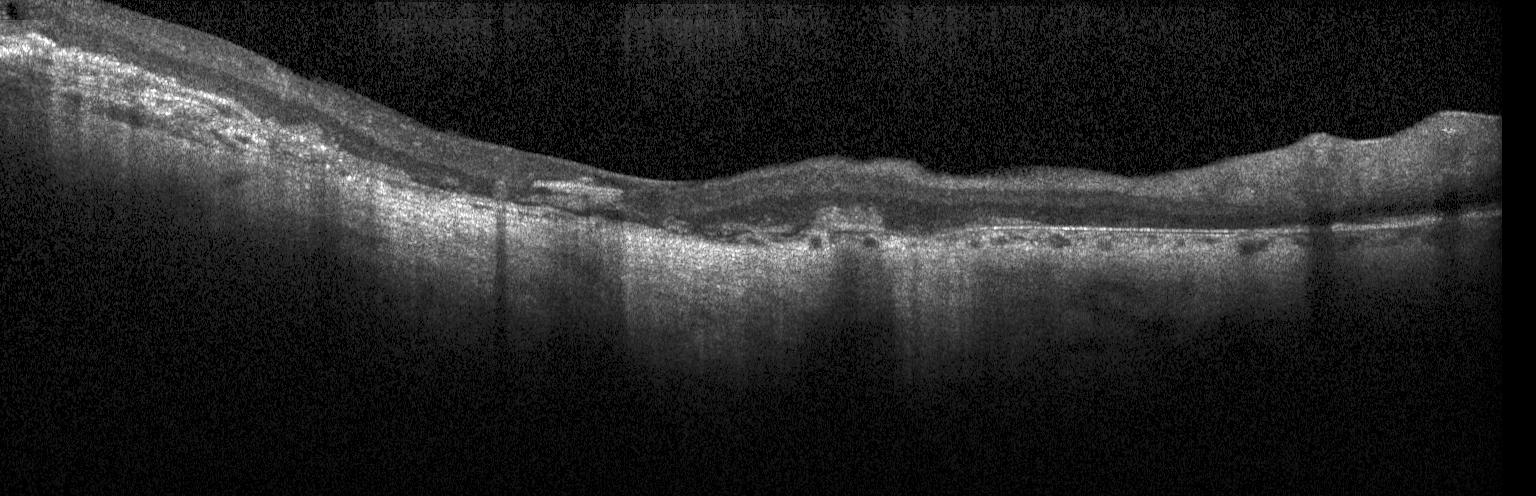 Choroidal neovascularization (CNV).